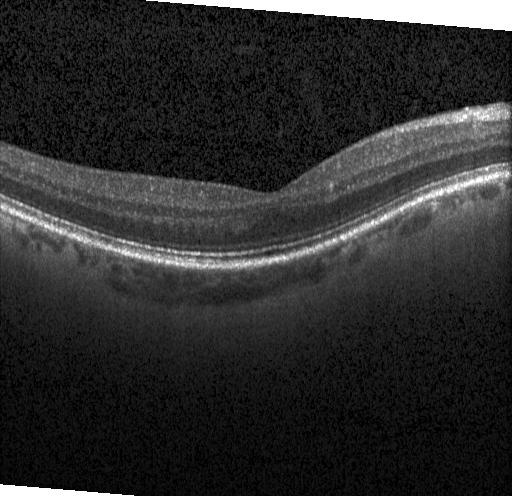

Finding: no evidence of choroidal neovascularization, diabetic macular edema, or drusen.